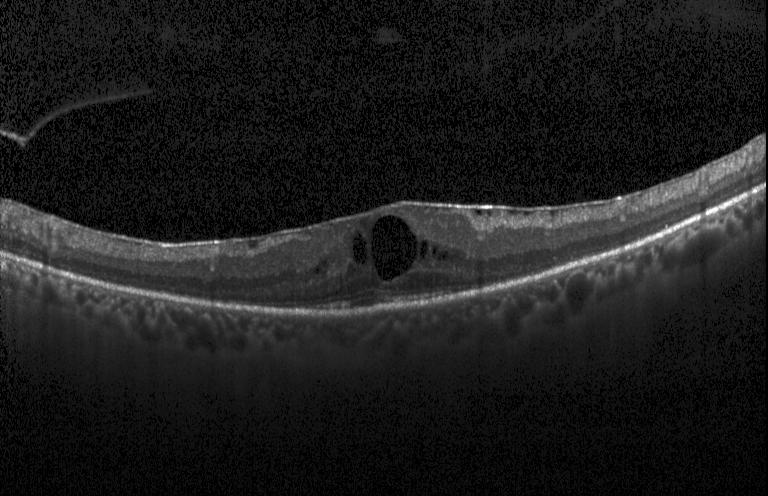

Retinal OCT cross-section showing diabetic macular edema.